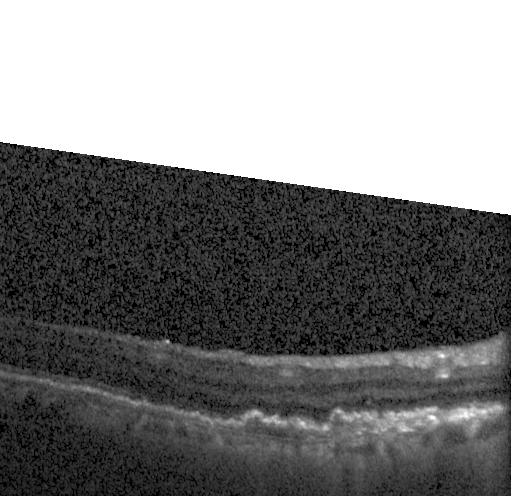

Impression: CNV.